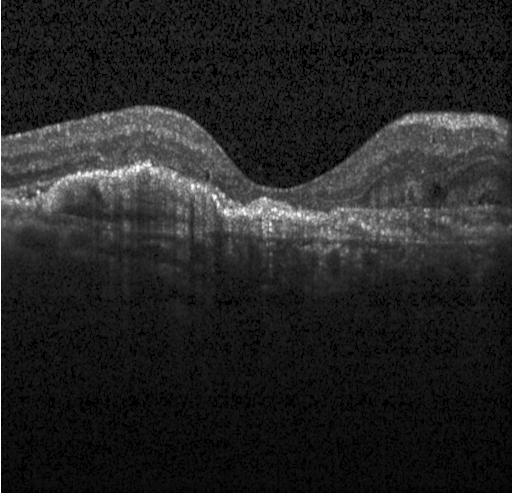 Retinal OCT B-scan; acquired on a Heidelberg Spectralis; fovea-centered
Finding: choroidal neovascularization.